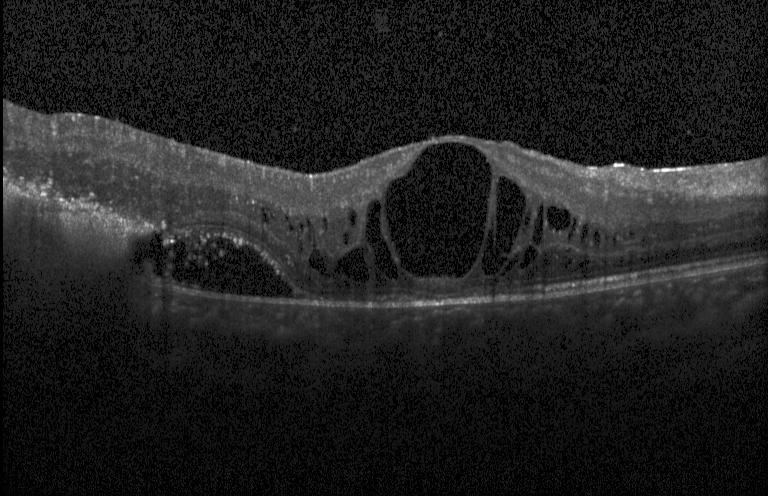
OCT scan showing diabetic macular edema (DME).